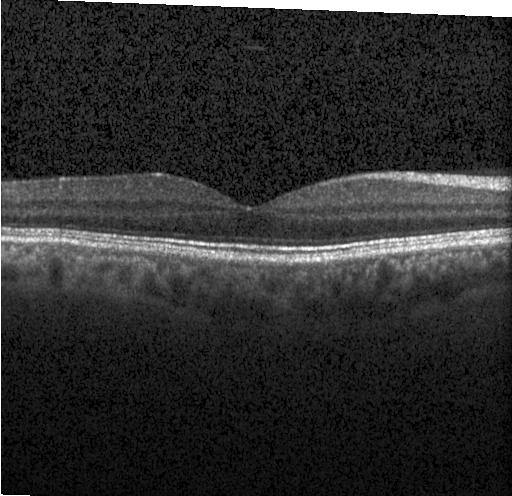

No evidence of CNV, DME, or drusen.